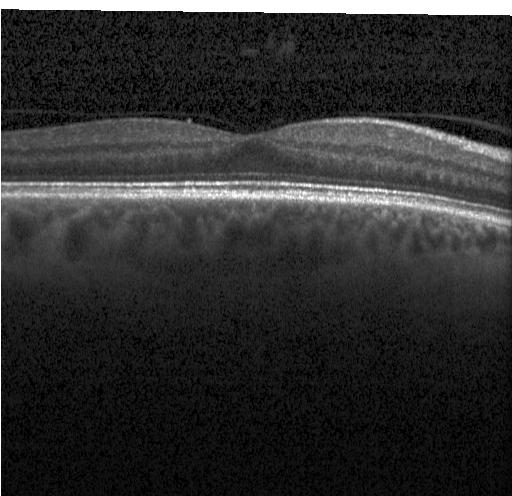
Optical coherence tomography scan
Macular OCT: neither choroidal neovascularization, diabetic macular edema, nor drusen.